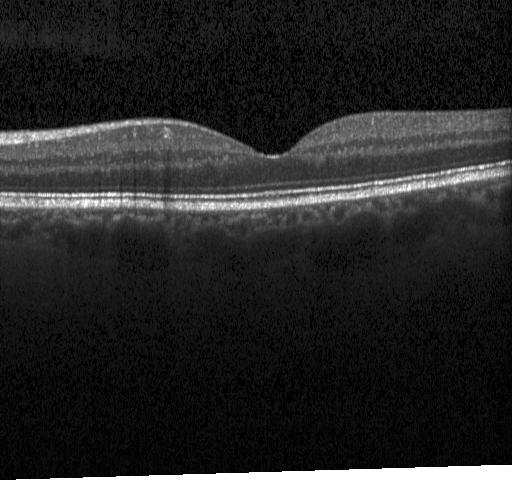
Finding: neither choroidal neovascularization, diabetic macular edema, nor drusen.